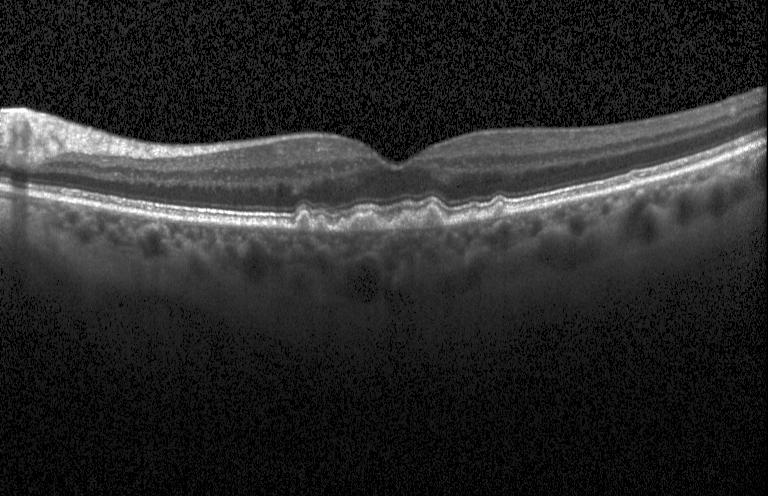
Through the macula, OCT B-scan, Heidelberg Spectralis. Impression: drusen.